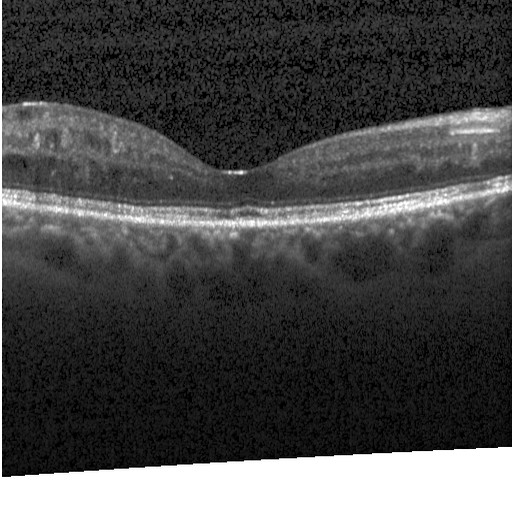

Instrument: Heidelberg Spectralis; optical coherence tomography scan.
OCT finding: diabetic macular edema (DME).